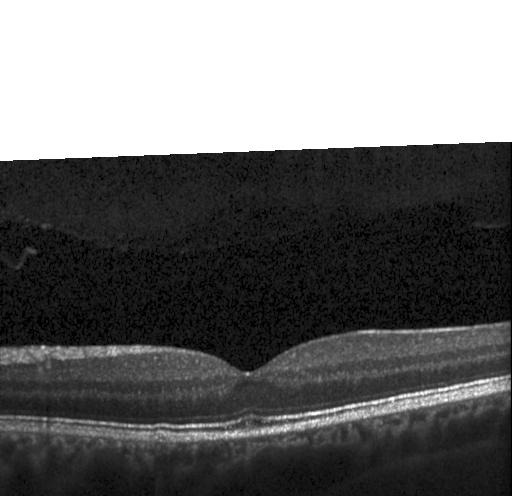

Optical coherence tomography scan · macular scan · spectral-domain OCT
OCT finding: no CNV, DME, or drusen.